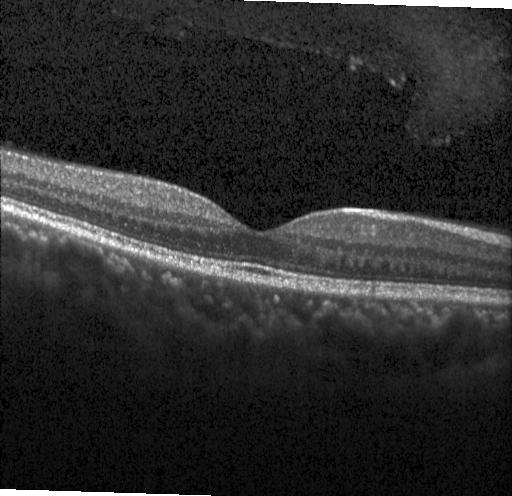
Impression: no evidence of choroidal neovascularization, diabetic macular edema, or drusen.